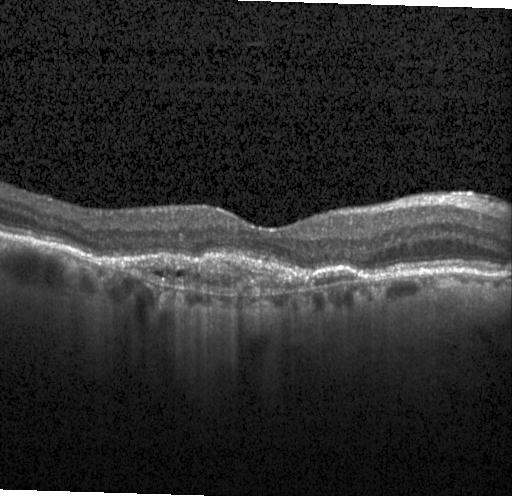

Centered on the fovea; spectral-domain optical coherence tomography; optical coherence tomography B-scan. Diagnosis: a choroidal neovascular membrane.